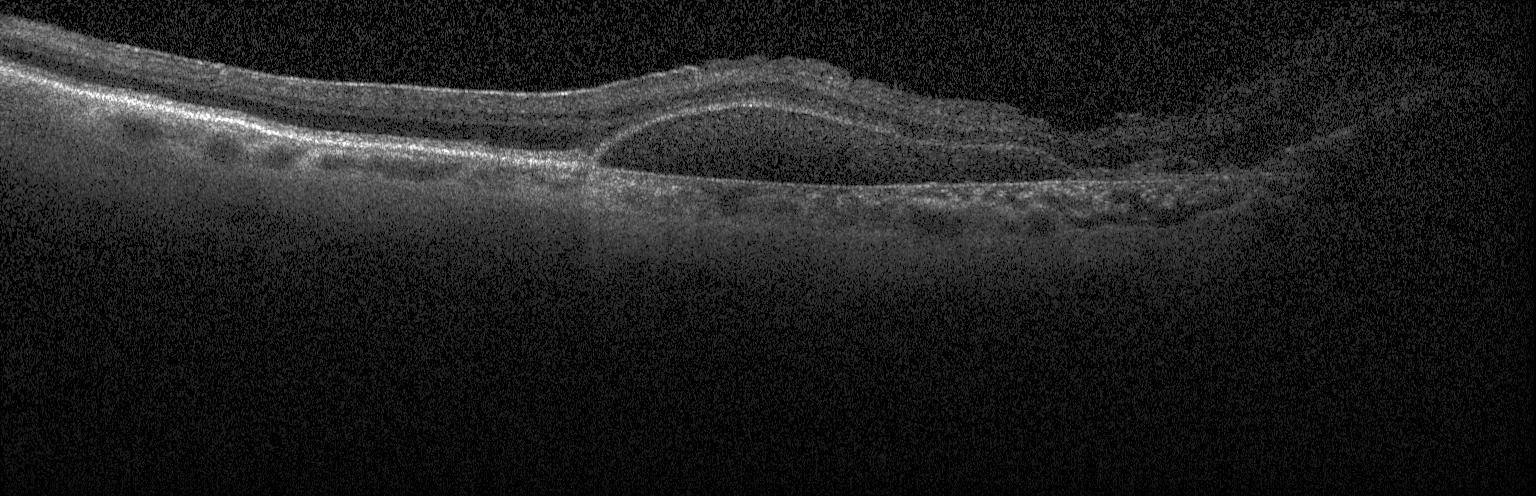 Assessment: choroidal neovascularization.